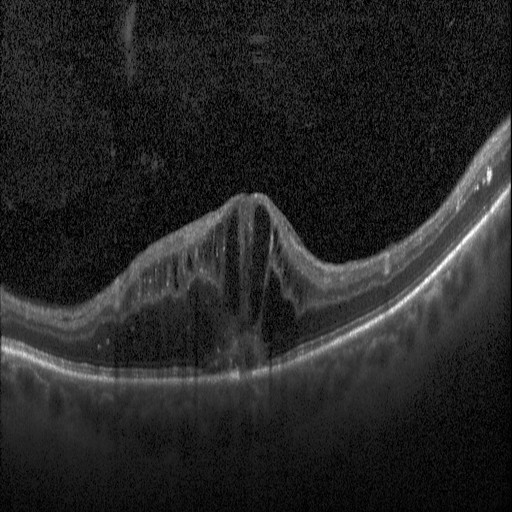
This B-scan demonstrates diabetic macular edema.